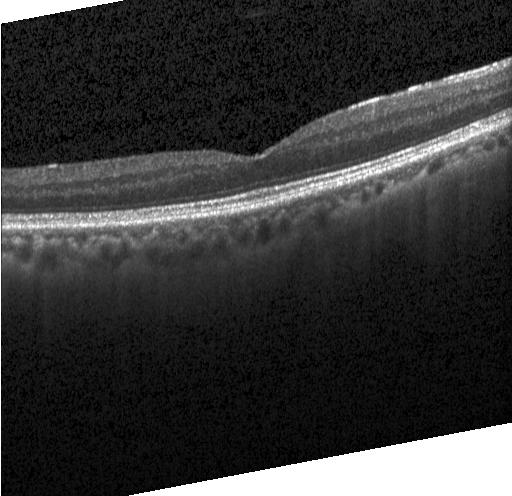
Heidelberg Spectralis OCT system. Retinal OCT B-scan. Spectral-domain optical coherence tomography. OCT finding: no evidence of choroidal neovascularization, diabetic macular edema, or drusen.